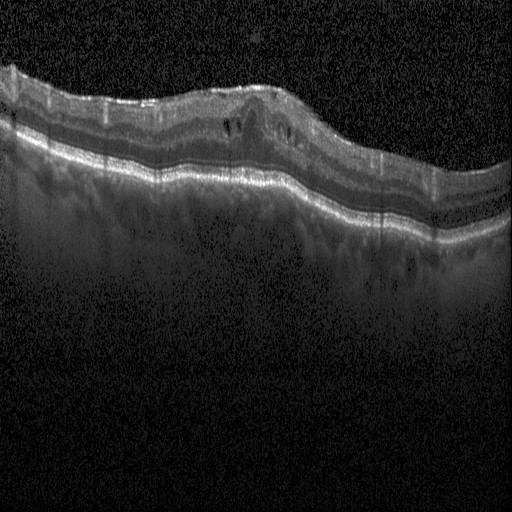

Instrument: Heidelberg Spectralis, OCT B-scan, fovea-centered, spectral-domain optical coherence tomography — DME.